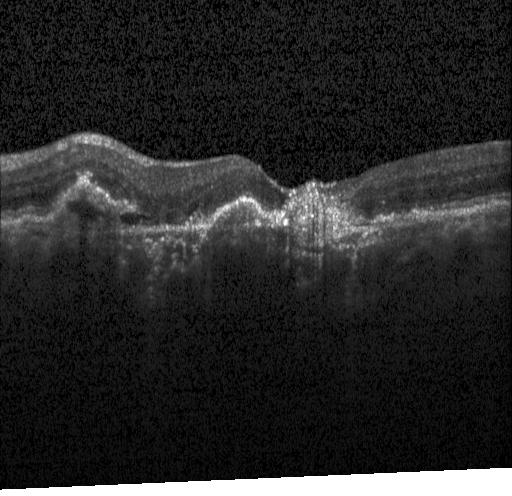
Optical coherence tomography B-scan — The scan shows choroidal neovascularization.